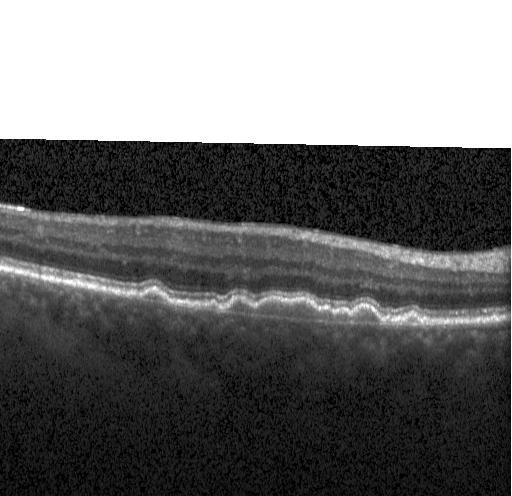

Impression: choroidal neovascularization.